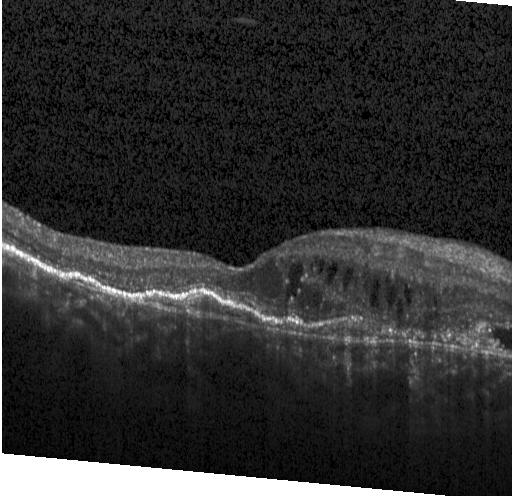
OCT finding: a choroidal neovascular membrane.